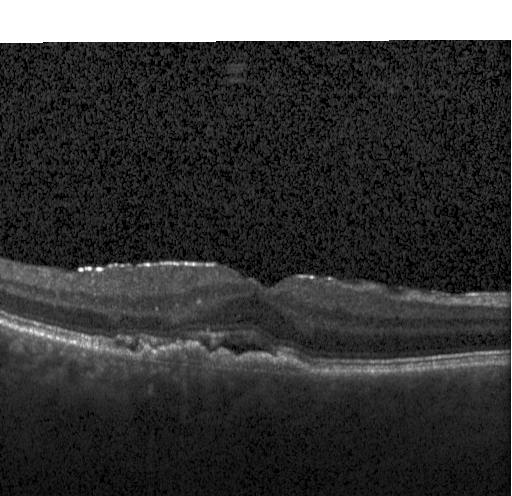

Through the macula. Optical coherence tomography scan.
CNV.